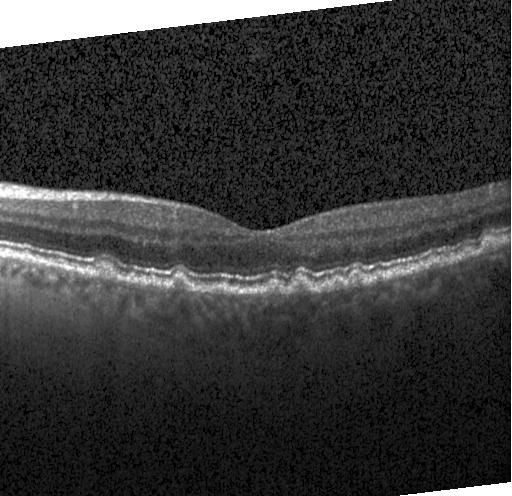
Finding: sub-RPE drusenoid deposits.